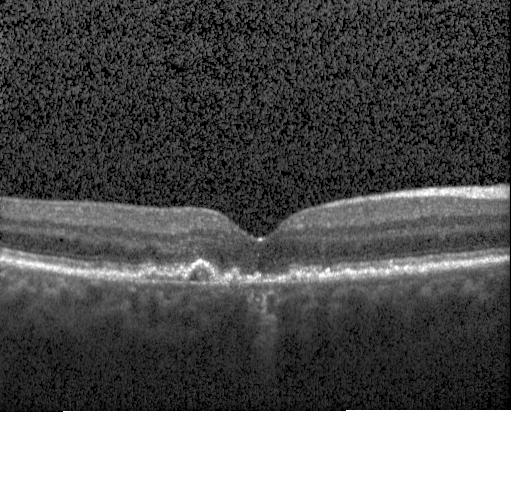

Optical coherence tomography B-scan, Heidelberg Spectralis, fovea-centered. This B-scan demonstrates choroidal neovascularization (CNV).